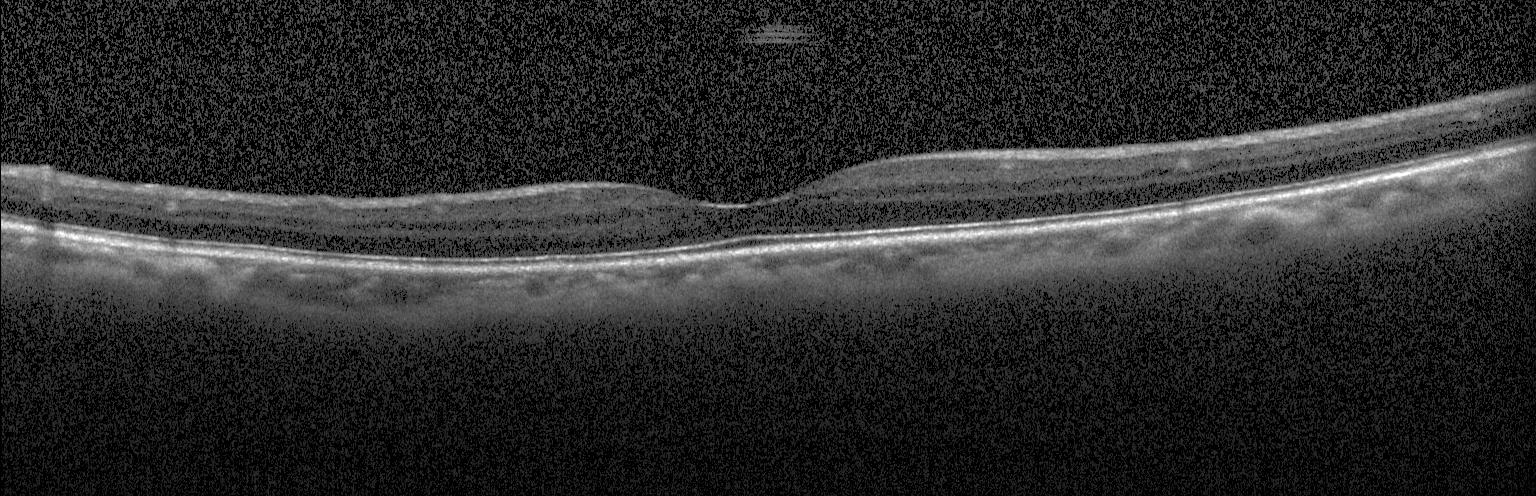 Diagnosis: no CNV, no DME, and no drusen.